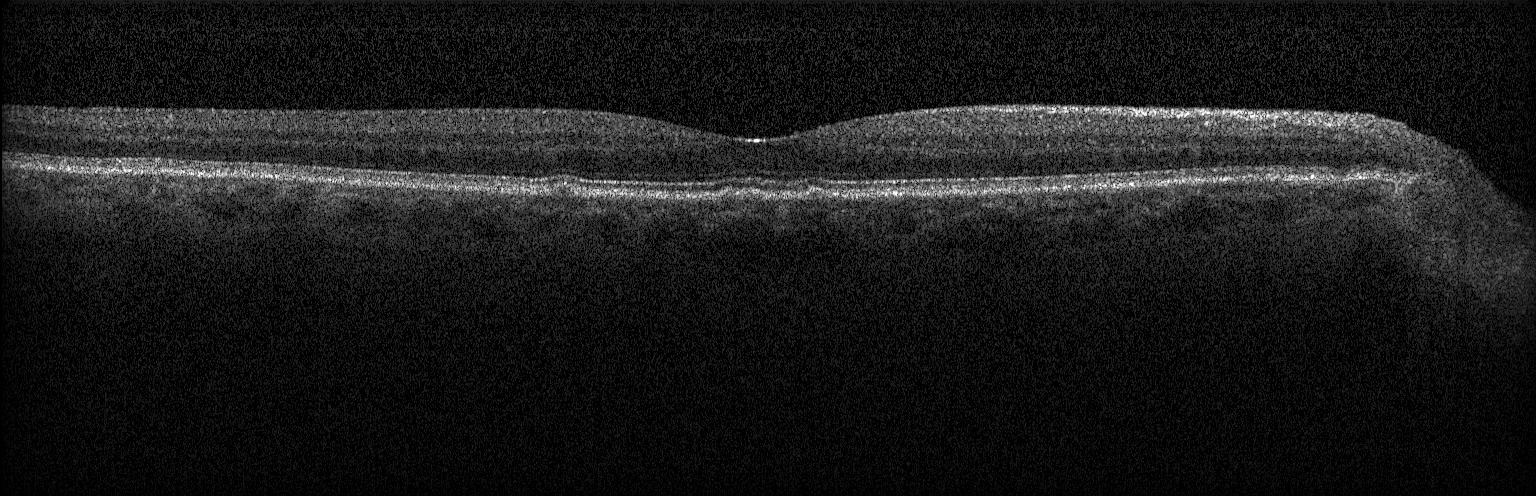 Through the macula · Heidelberg Spectralis · OCT B-scan — Finding: multiple drusen.